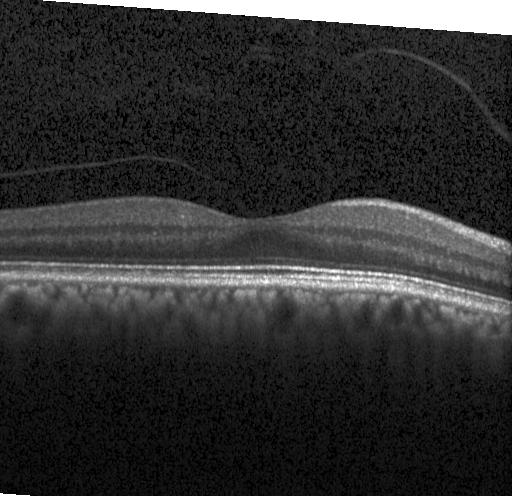
OCT B-scan showing neither choroidal neovascularization, diabetic macular edema, nor drusen.